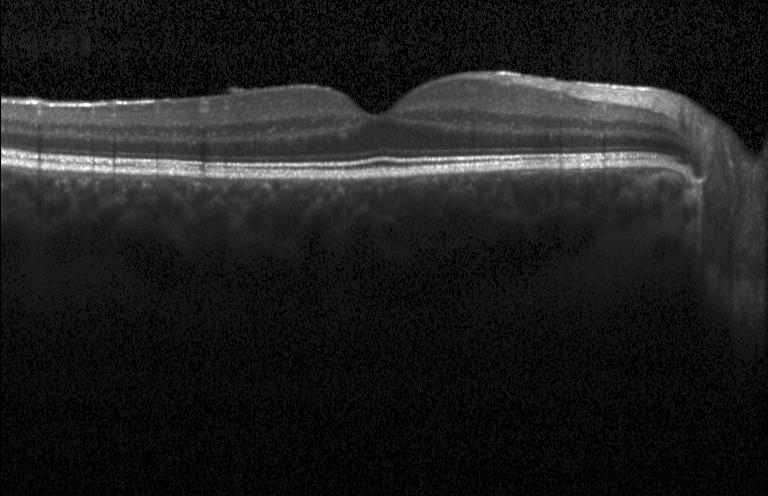
Through the macula, OCT B-scan, SD-OCT, Heidelberg Spectralis
Assessment: no evidence of choroidal neovascularization, diabetic macular edema, or drusen.